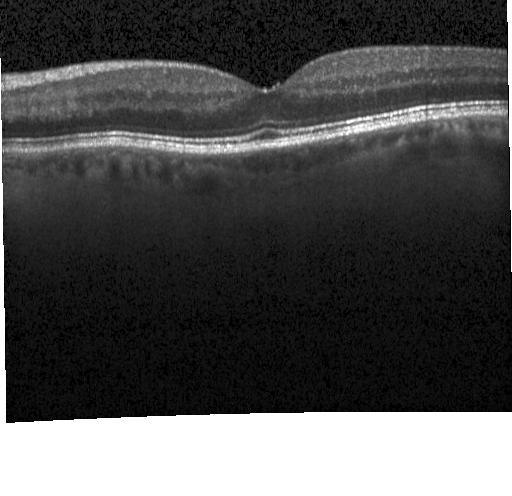 Spectral-domain optical coherence tomography · retinal OCT cross-section · Heidelberg Spectralis OCT system · horizontal scan through the fovea. Macular OCT: no evidence of choroidal neovascularization, diabetic macular edema, or drusen.